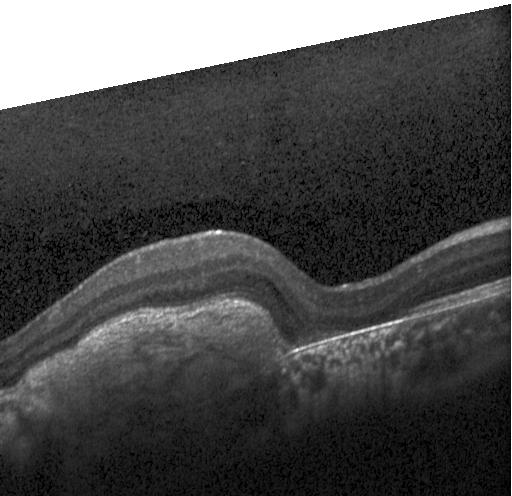 Assessment: a choroidal neovascular membrane.